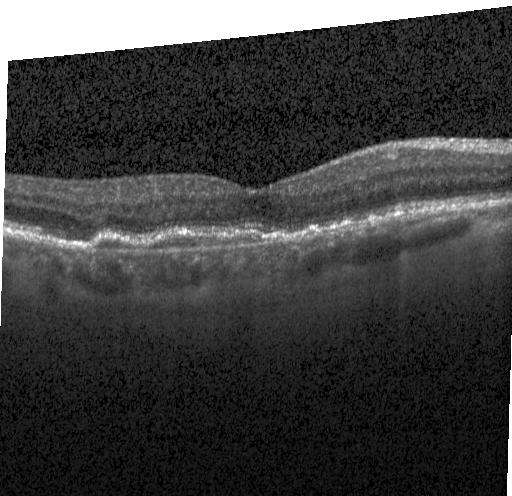
OCT B-scan showing a choroidal neovascular membrane.